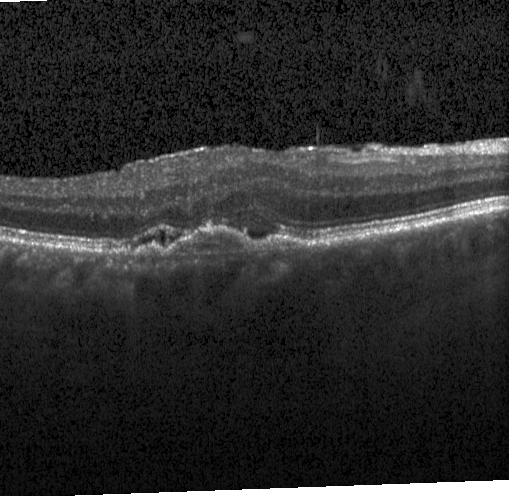 Heidelberg Spectralis OCT system · spectral-domain optical coherence tomography · centered on the fovea · OCT B-scan.
Dx: CNV.